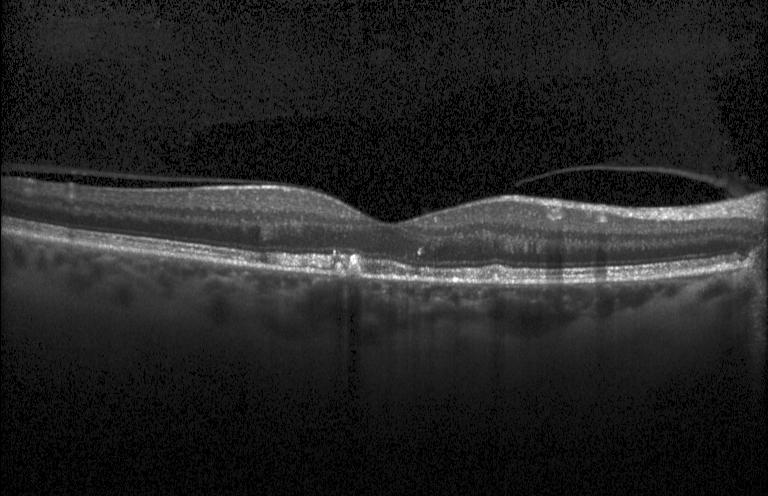

SD-OCT. Retinal OCT B-scan. Impression: multiple drusen.